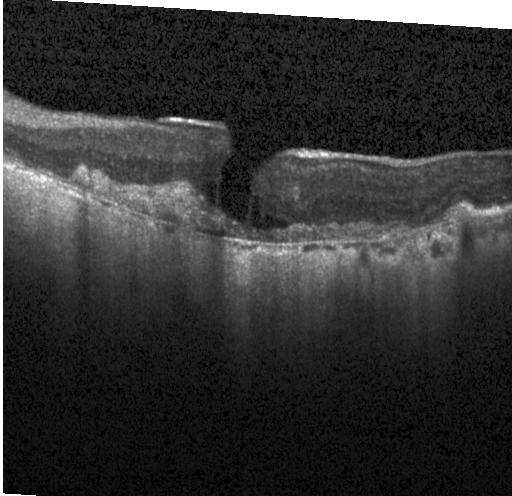 Macular OCT: choroidal neovascularization.